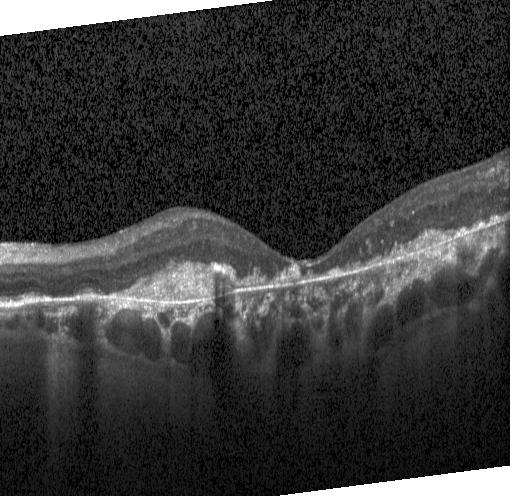 Through the macula; optical coherence tomography scan
Assessment: a choroidal neovascular membrane.